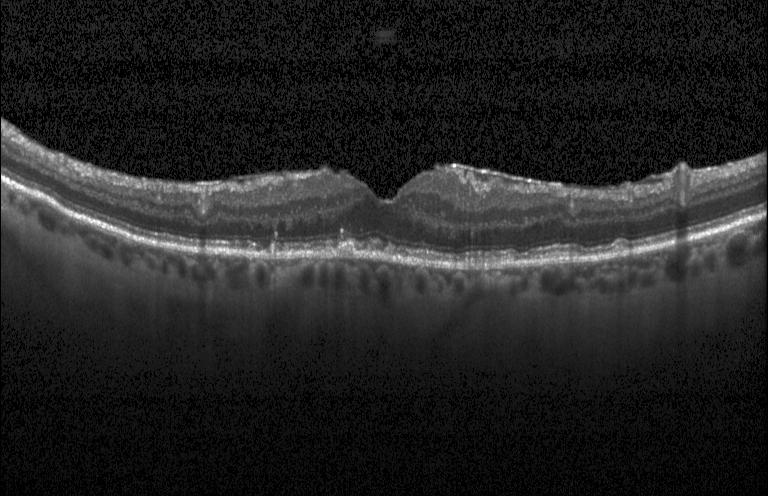
Heidelberg Spectralis OCT system; optical coherence tomography B-scan. The scan shows drusen.